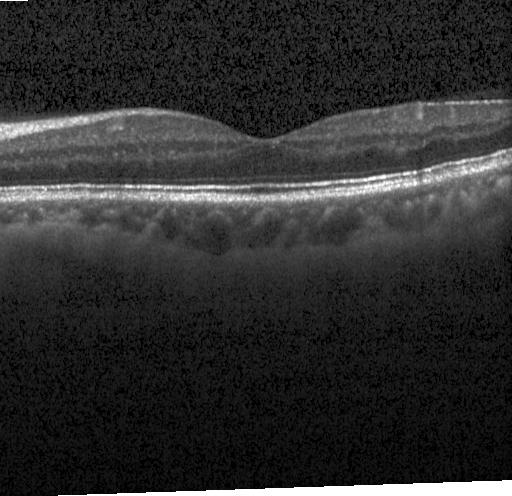

Impression: neither CNV, DME, nor drusen.